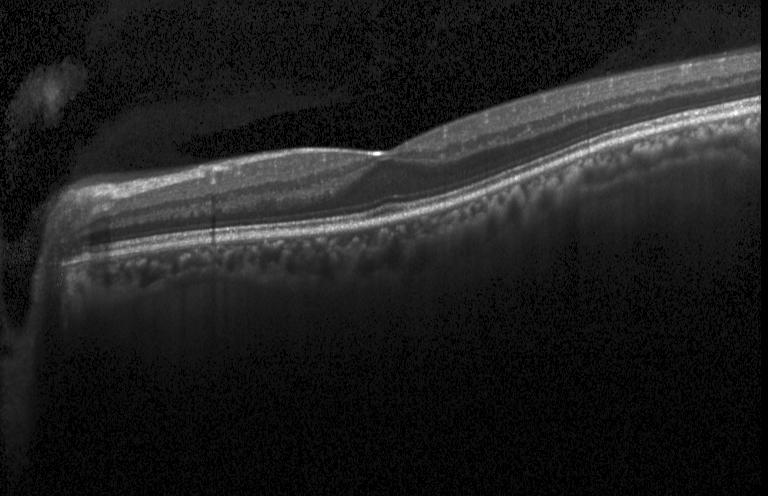
Macular scan, OCT B-scan — Impression: no CNV, DME, or drusen.